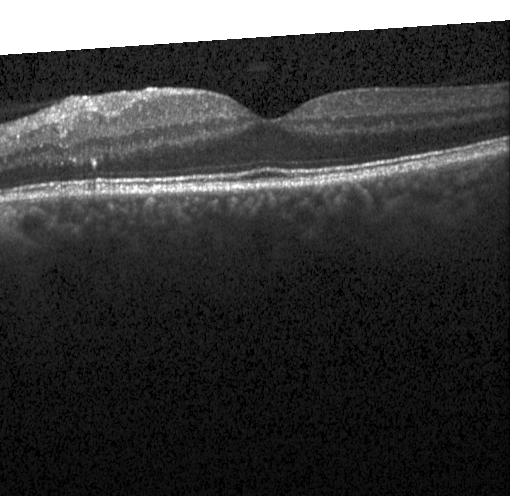 Retinal OCT cross-section showing no evidence of choroidal neovascularization, diabetic macular edema, or drusen.